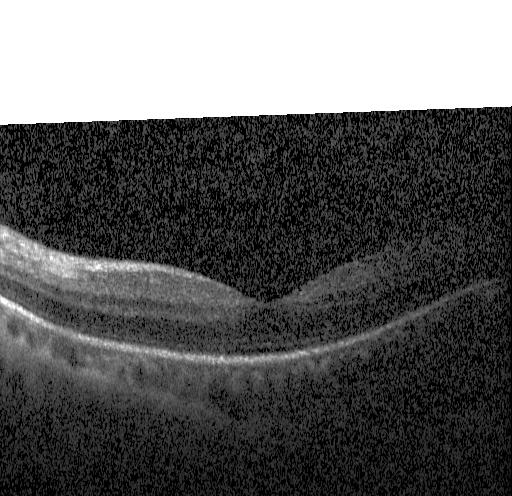

OCT B-scan — Diagnosis: no choroidal neovascularization, no diabetic macular edema, and no drusen.